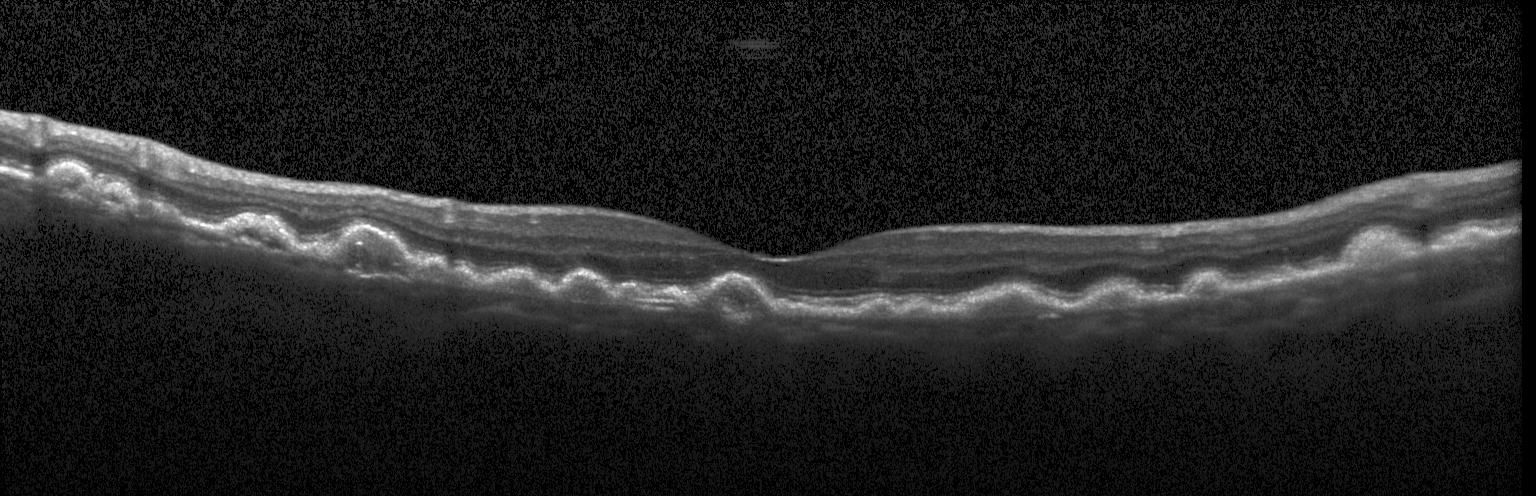 Optical coherence tomography B-scan. SD-OCT. Fovea-centered. Acquired on a Heidelberg Spectralis — Finding: multiple drusen.